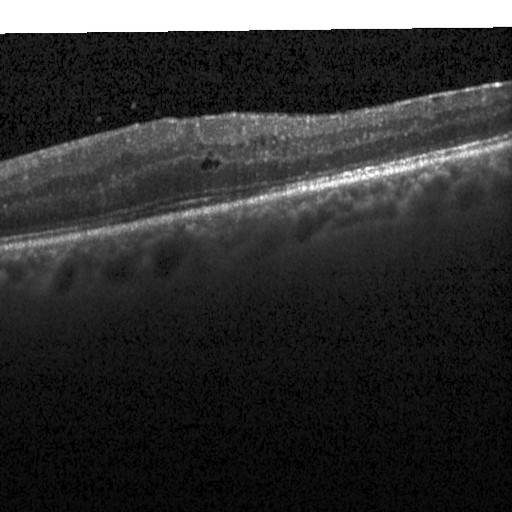

OCT line scan. Diabetic macular edema (DME).